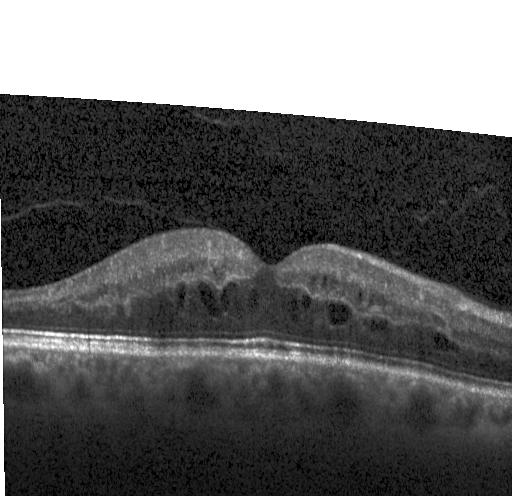 Macular scan; instrument: Heidelberg Spectralis; OCT B-scan. Impression: diabetic macular edema.